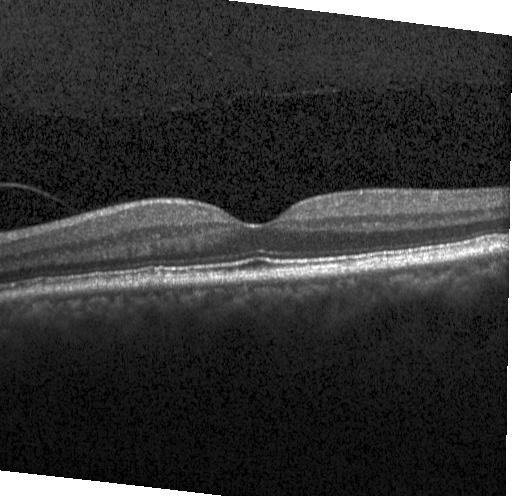

OCT finding: no evidence of choroidal neovascularization, diabetic macular edema, or drusen.